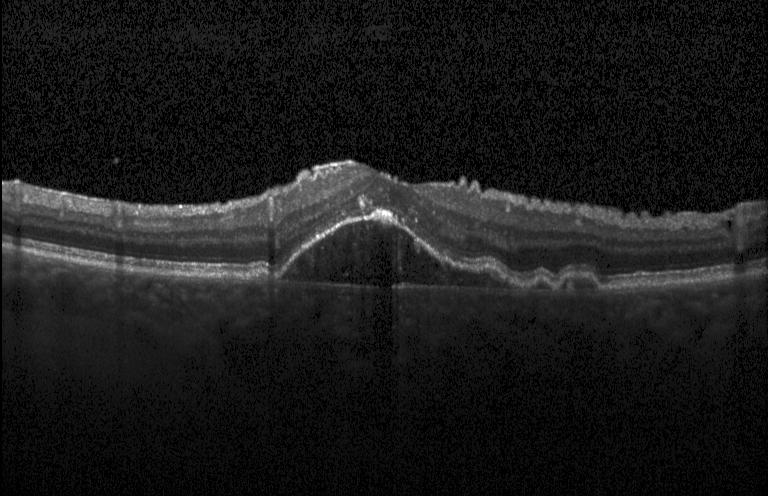
Impression: choroidal neovascularization (CNV).